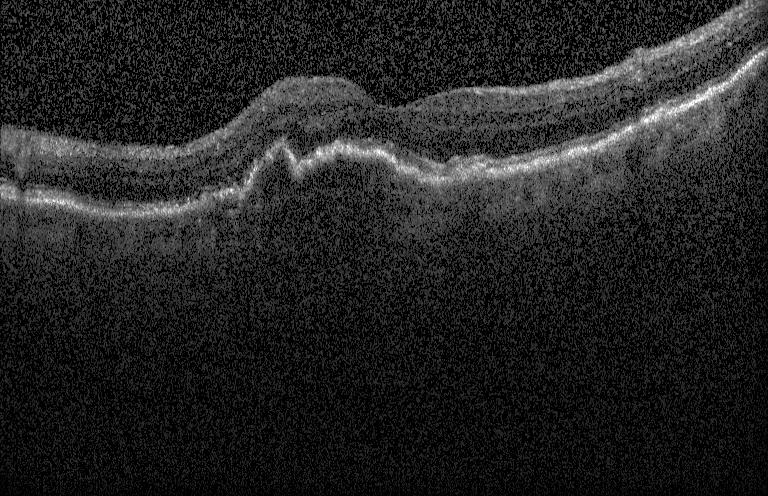

Horizontal scan through the fovea; Heidelberg Spectralis; retinal OCT B-scan. Diagnosis: choroidal neovascularization.